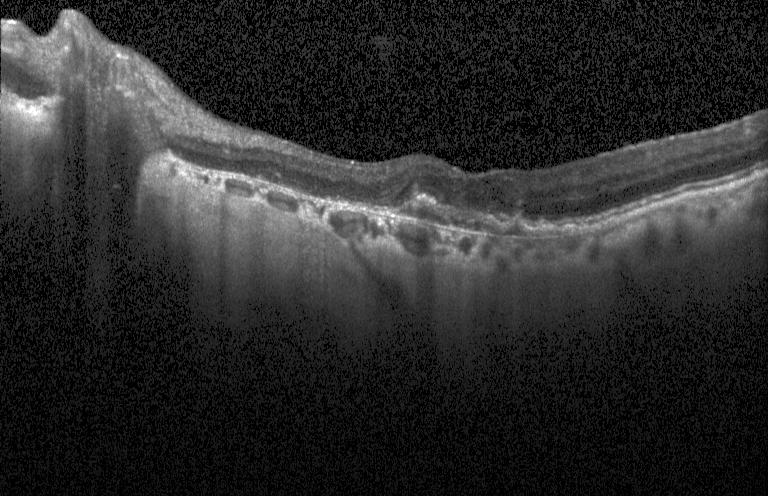 OCT finding: CNV.